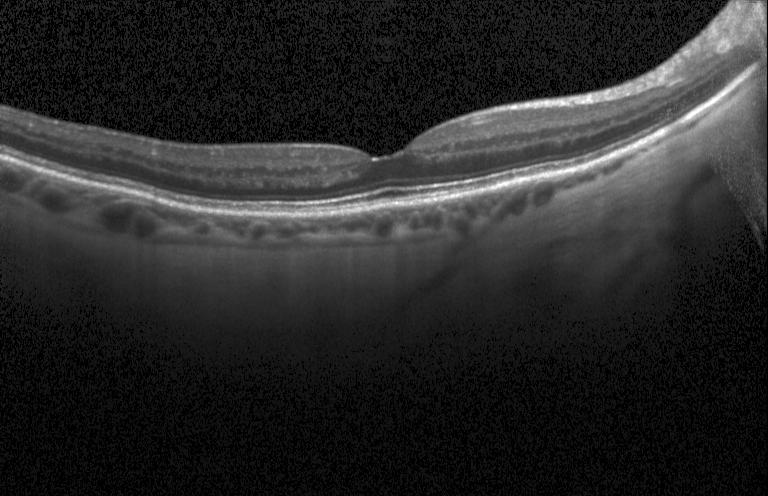

OCT finding: neither choroidal neovascularization, diabetic macular edema, nor drusen.